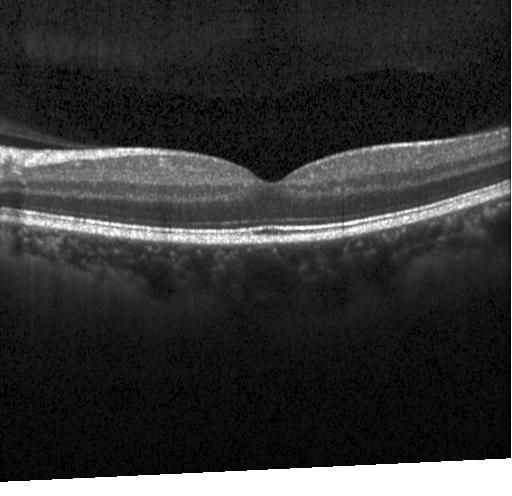

Retinal OCT cross-section · centered on the fovea · acquired on a Heidelberg Spectralis · spectral-domain OCT — No CNV, DME, or drusen.